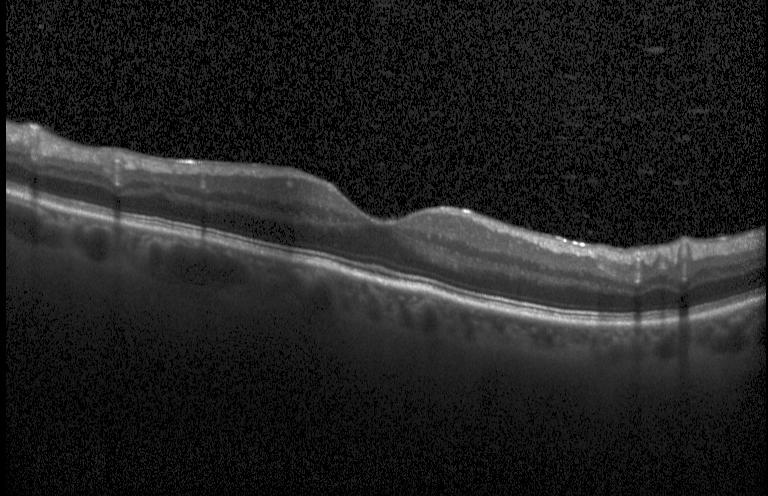

Optical coherence tomography B-scan
The scan shows no choroidal neovascularization, no diabetic macular edema, and no drusen.